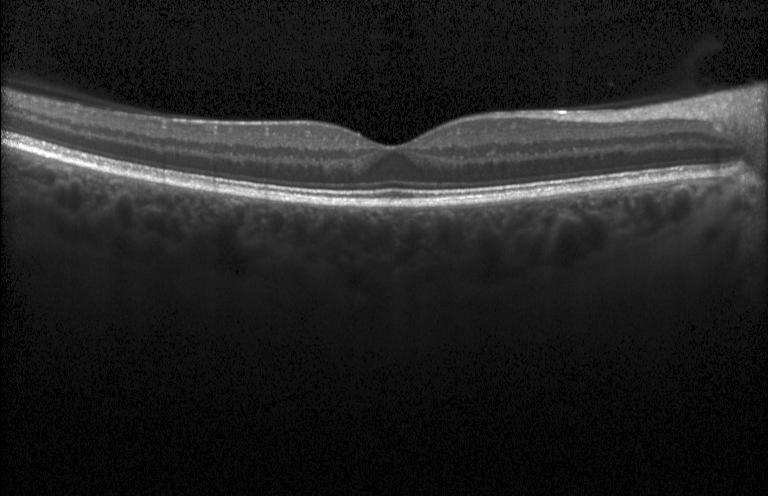
Diagnosis: no evidence of choroidal neovascularization, diabetic macular edema, or drusen.